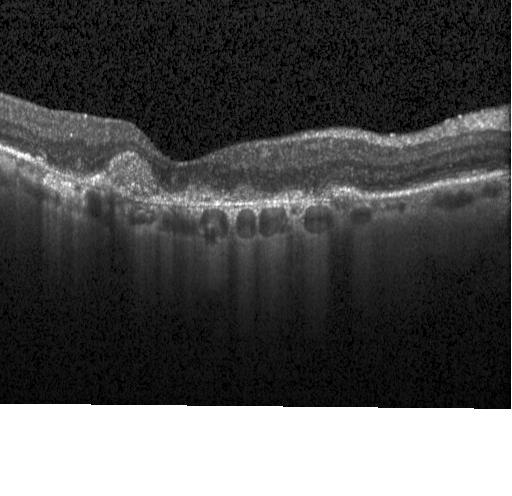
SD-OCT; OCT B-scan.
Assessment: choroidal neovascularization.